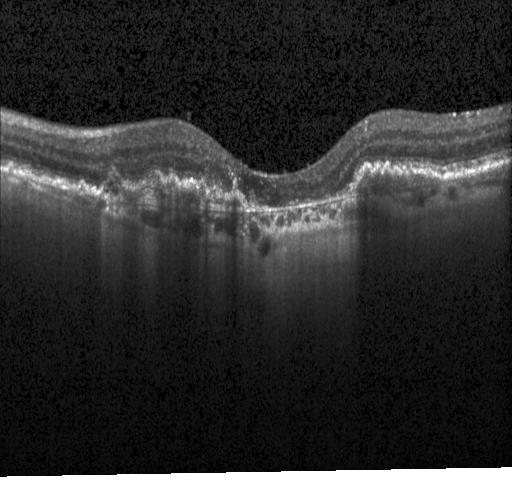
This B-scan demonstrates a choroidal neovascular membrane.